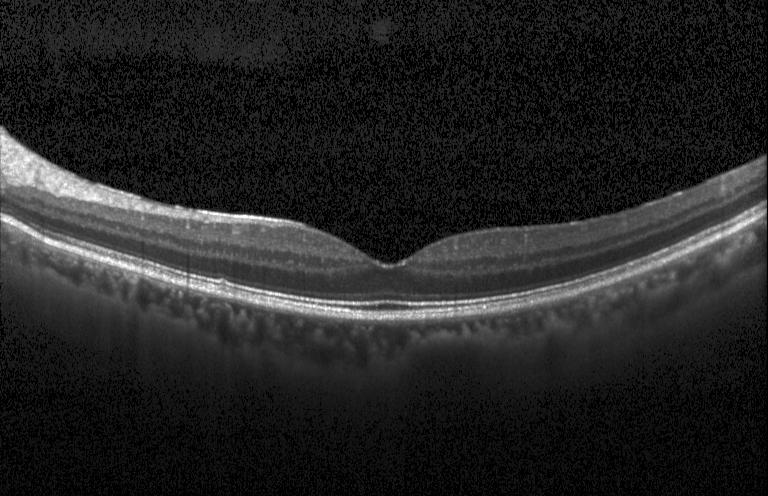

Optical coherence tomography scan, spectral-domain optical coherence tomography. OCT finding: neither CNV, DME, nor drusen.